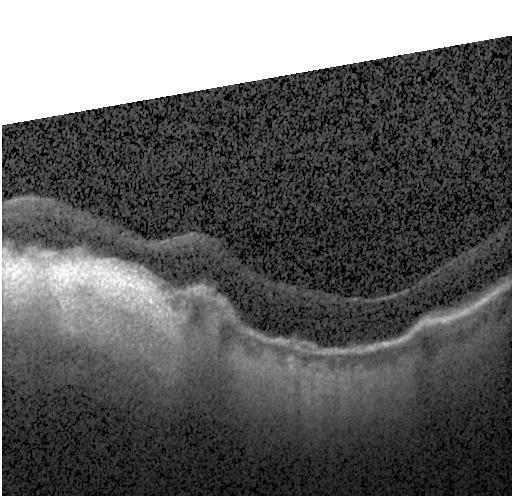
Heidelberg Spectralis; retinal OCT B-scan; horizontal scan through the fovea; SD-OCT — Finding: a choroidal neovascular membrane.